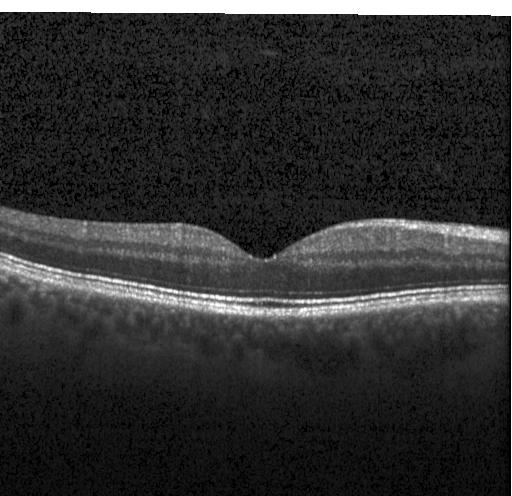

Diagnosis: neither CNV, DME, nor drusen.